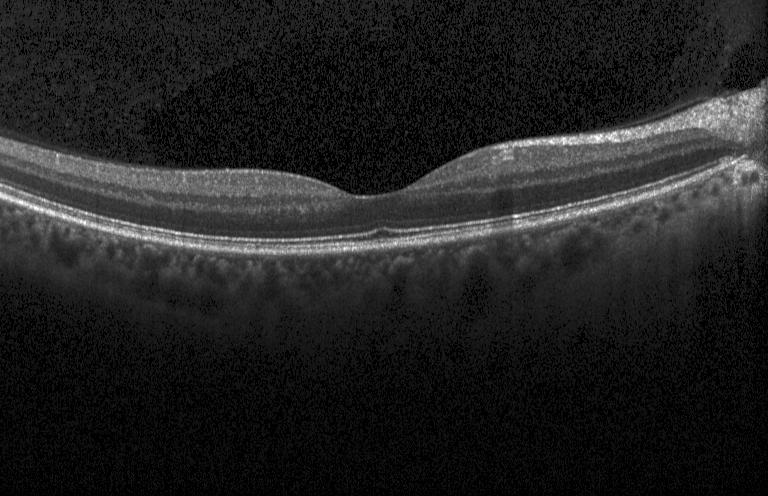 Horizontal scan through the fovea · spectral-domain optical coherence tomography · retinal OCT cross-section.
Diagnosis: no choroidal neovascularization, no diabetic macular edema, and no drusen.